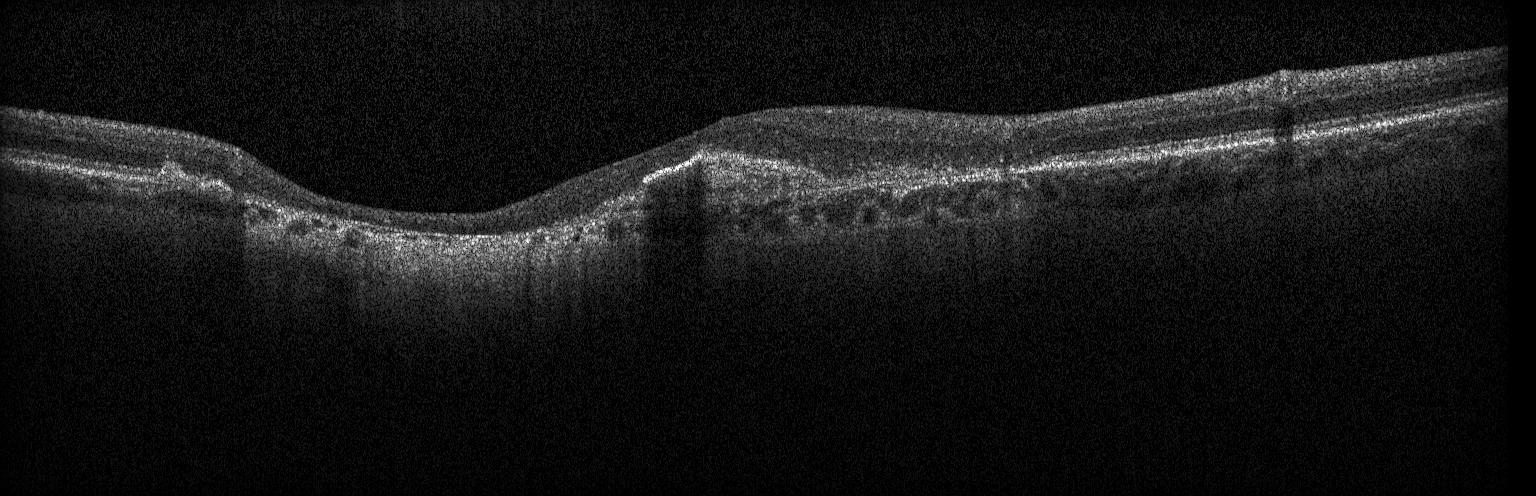 Heidelberg Spectralis. Optical coherence tomography scan. Fovea-centered. Spectral-domain optical coherence tomography. Diagnosis: a choroidal neovascular membrane.